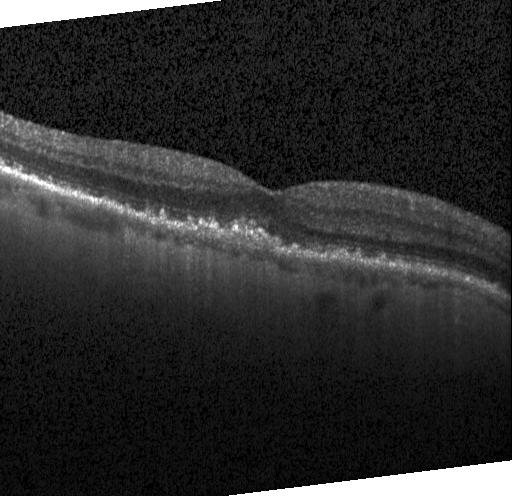
Sub-RPE drusenoid deposits.